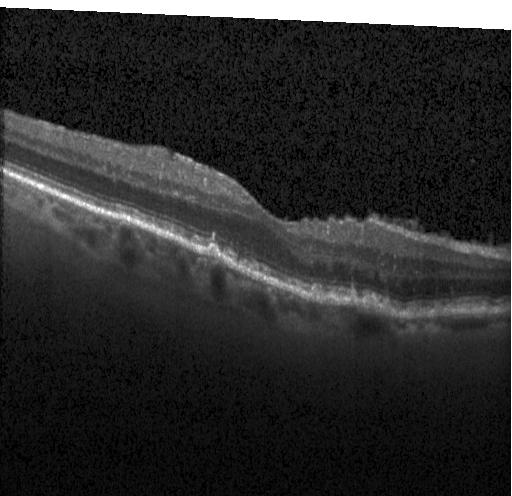

OCT line scan — The scan shows drusen.